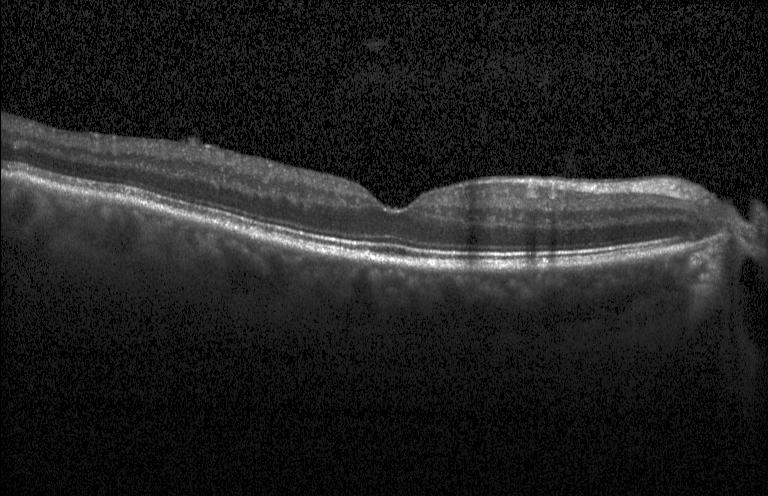 Finding: neither choroidal neovascularization, diabetic macular edema, nor drusen.